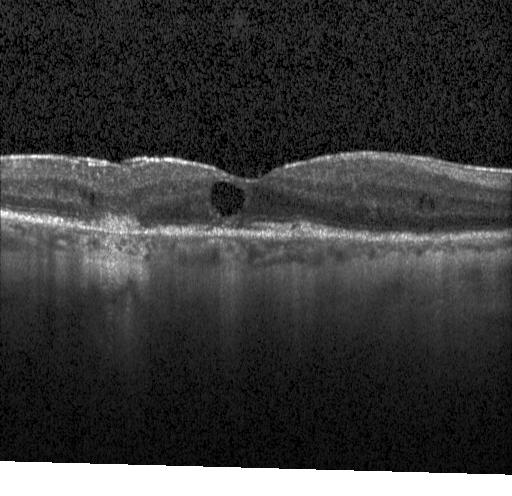

Finding: choroidal neovascularization (CNV).